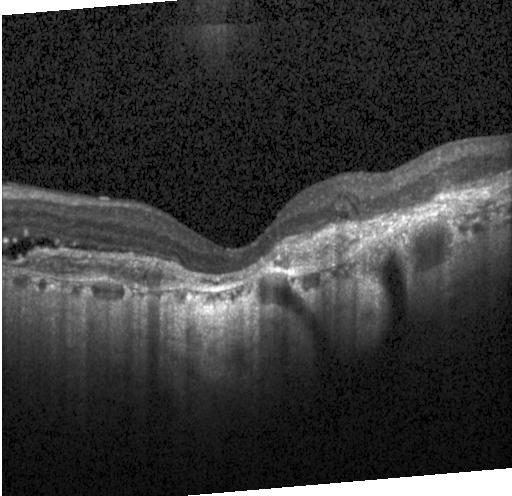
Finding: CNV.